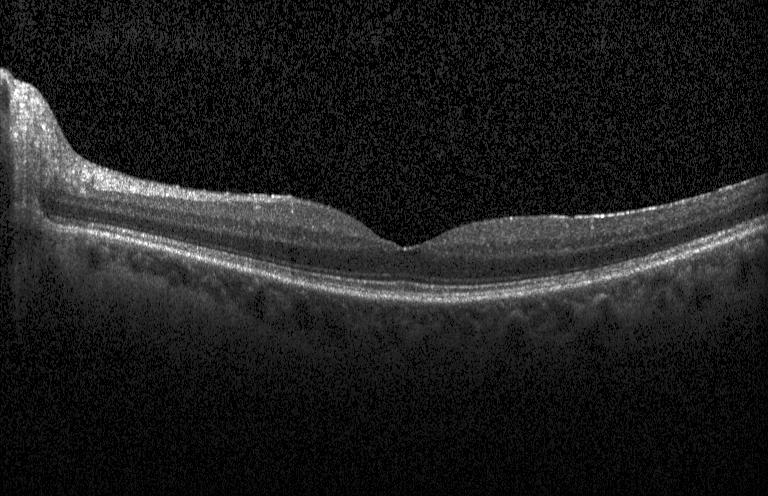
Acquired on a Heidelberg Spectralis. Through the macula. Optical coherence tomography B-scan. Spectral-domain optical coherence tomography
Diagnosis: no choroidal neovascularization, no diabetic macular edema, and no drusen.